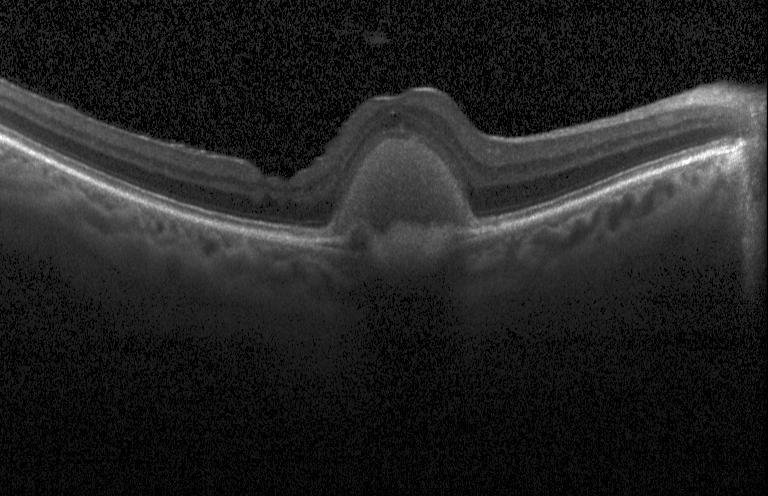
Diagnosis: CNV.